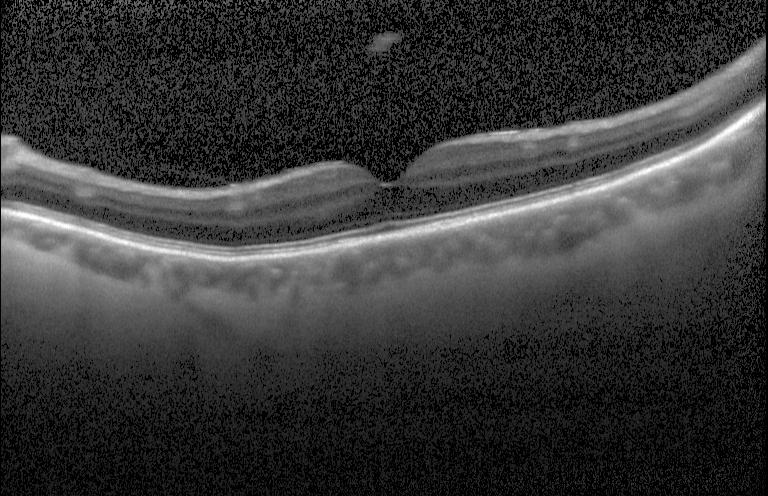
Spectral-domain optical coherence tomography, macular scan, OCT line scan, Heidelberg Spectralis. Diagnosis: no choroidal neovascularization, no diabetic macular edema, and no drusen.